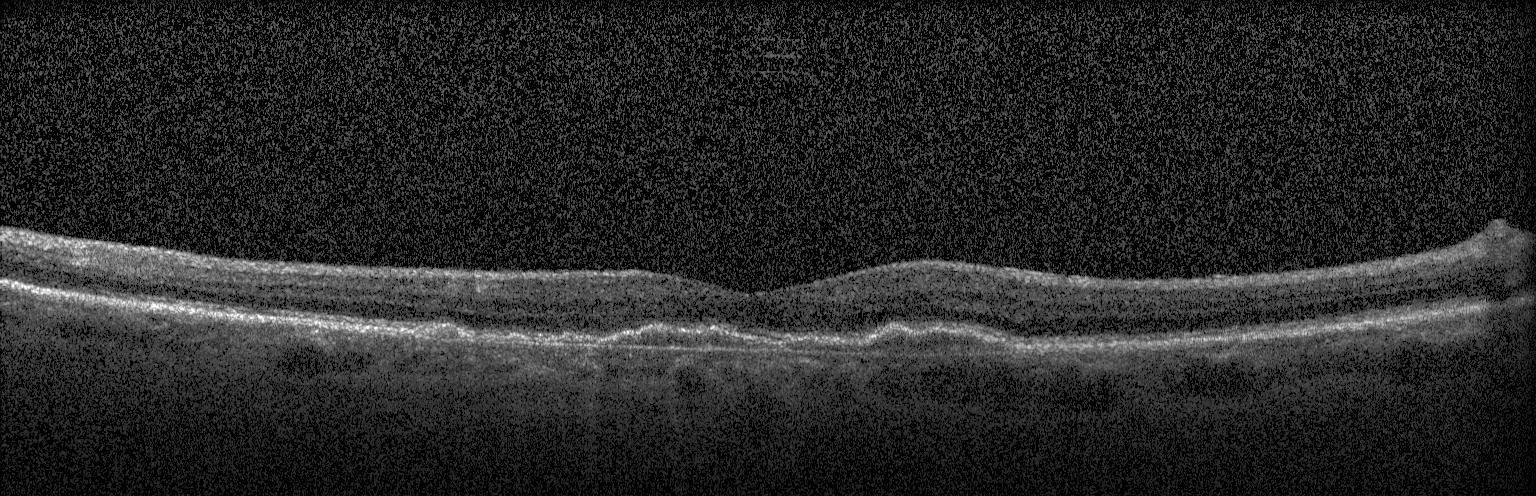

Optical coherence tomography B-scan, acquired on a Heidelberg Spectralis.
Dx: CNV.